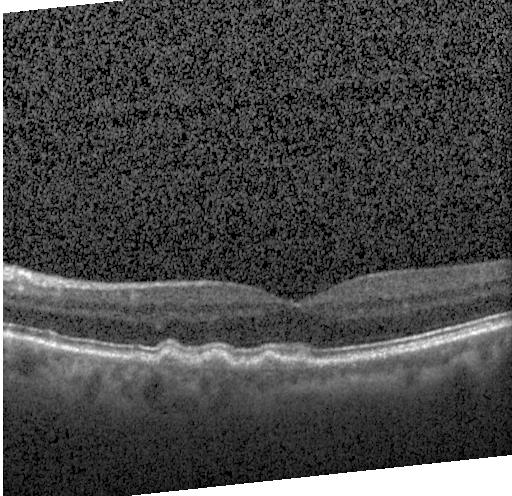

Finding: sub-RPE drusenoid deposits.